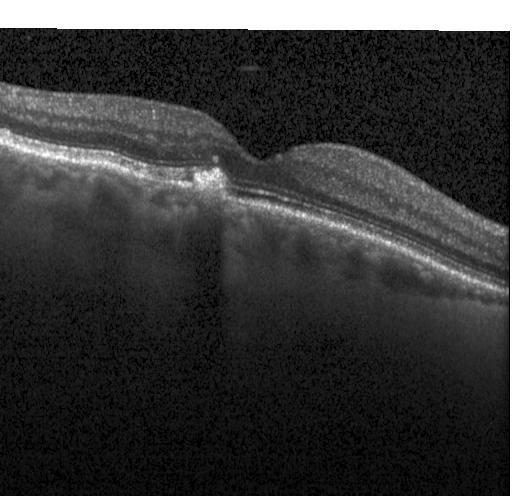

Retinal OCT B-scan, spectral-domain OCT — This B-scan demonstrates multiple drusen.